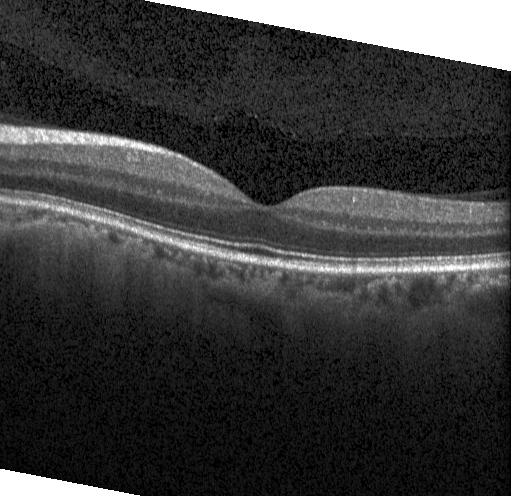

OCT B-scan — Finding: neither choroidal neovascularization, diabetic macular edema, nor drusen.